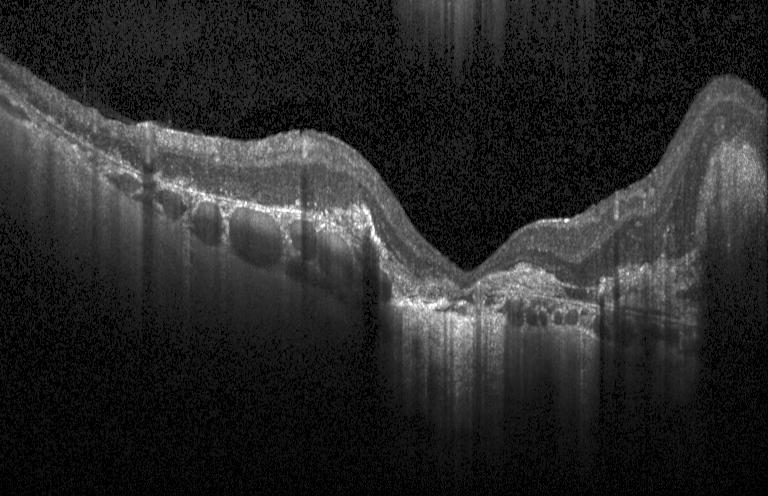
OCT finding: a choroidal neovascular membrane.